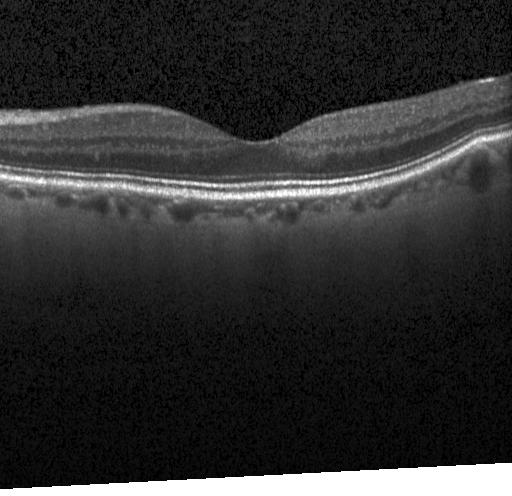 SD-OCT; optical coherence tomography B-scan. The scan shows no CNV, no DME, and no drusen.